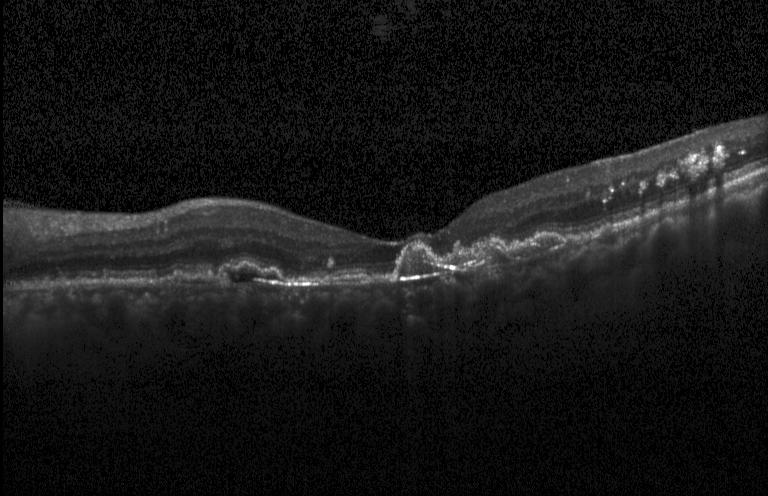 Horizontal scan through the fovea · OCT B-scan · SD-OCT · instrument: Heidelberg Spectralis
Finding: a choroidal neovascular membrane.